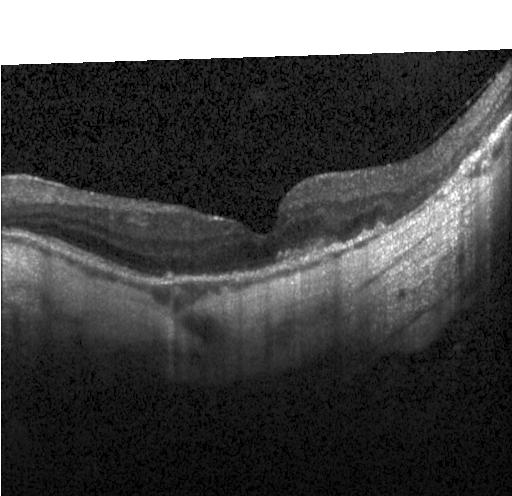

Optical coherence tomography B-scan · through the macula. Diagnosis: choroidal neovascularization.